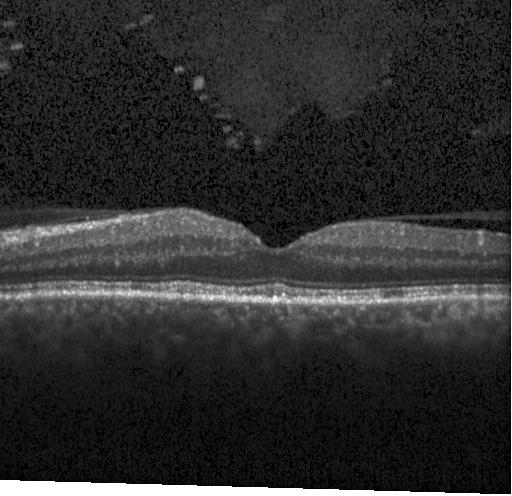

Instrument: Heidelberg Spectralis; OCT line scan; spectral-domain OCT; centered on the fovea
Finding: sub-RPE drusenoid deposits.